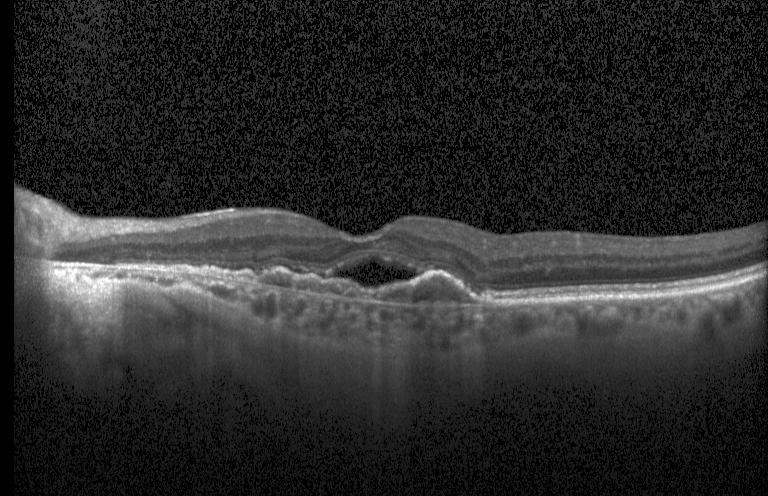

Finding: a choroidal neovascular membrane.